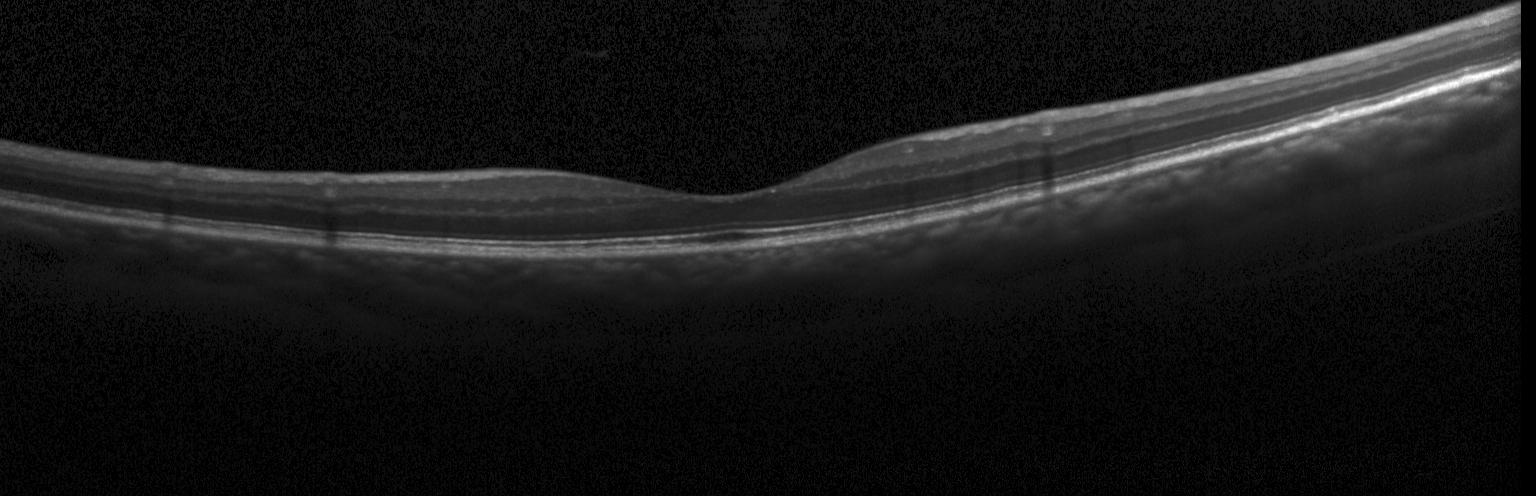
This B-scan demonstrates no CNV, no DME, and no drusen.